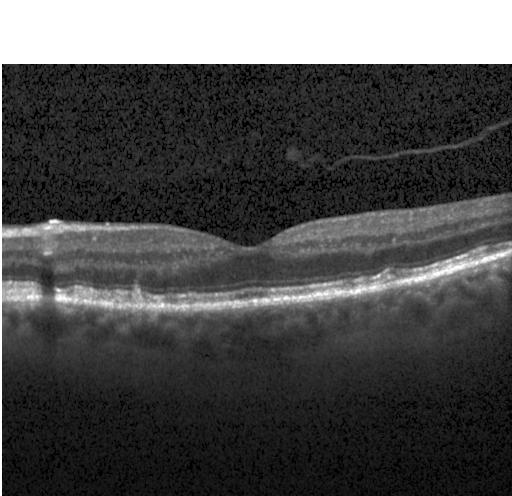
OCT line scan — The scan shows multiple drusen.